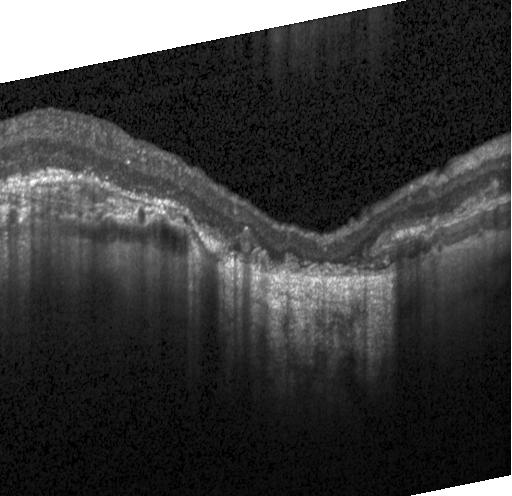

Diagnosis: CNV.